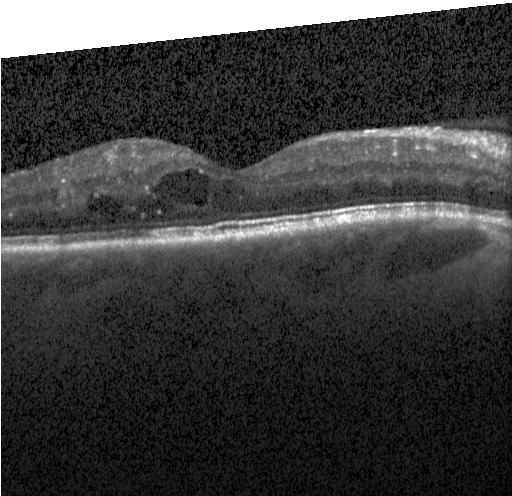 Horizontal scan through the fovea, OCT line scan. OCT finding: DME.